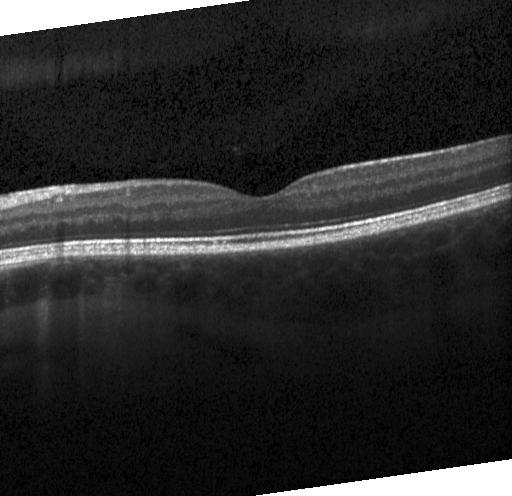
Centered on the fovea; OCT B-scan; spectral-domain optical coherence tomography.
This B-scan demonstrates neither CNV, DME, nor drusen.